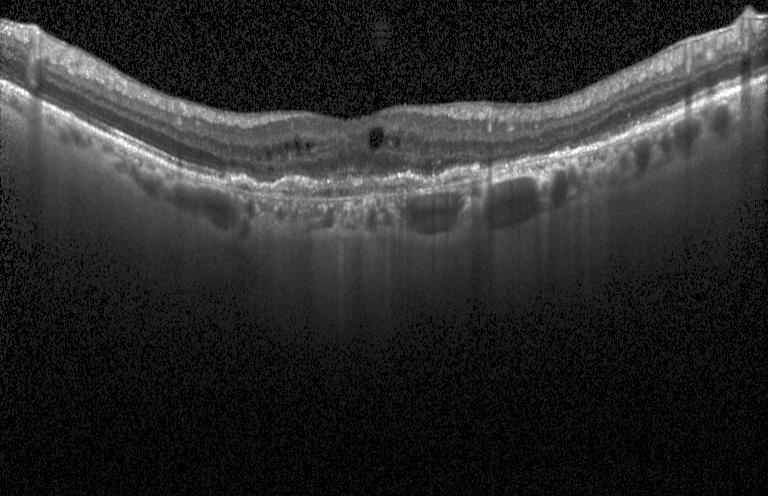 Heidelberg Spectralis OCT system, retinal OCT B-scan
Diagnosis: choroidal neovascularization.